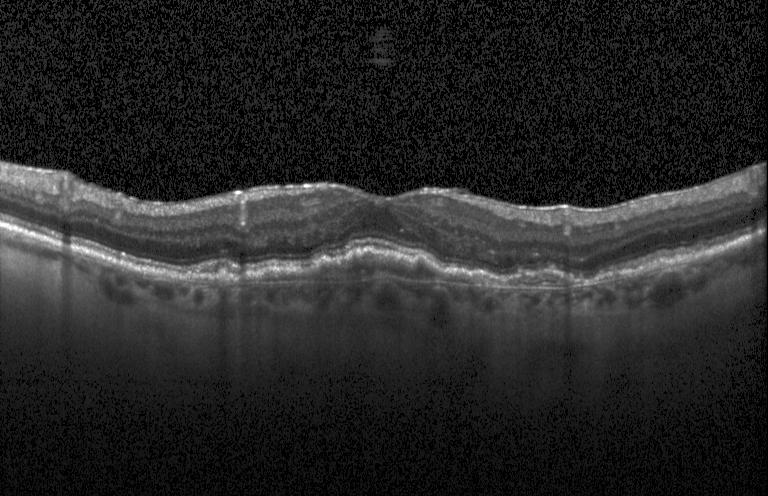
Impression: CNV.